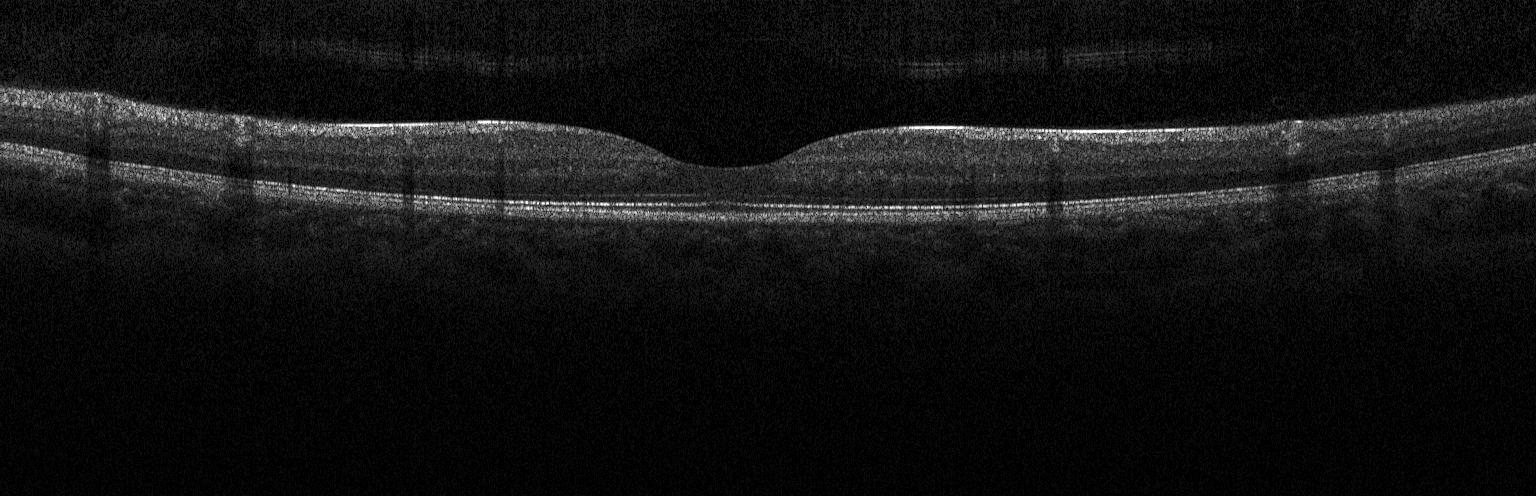

Dx: no evidence of choroidal neovascularization, diabetic macular edema, or drusen.